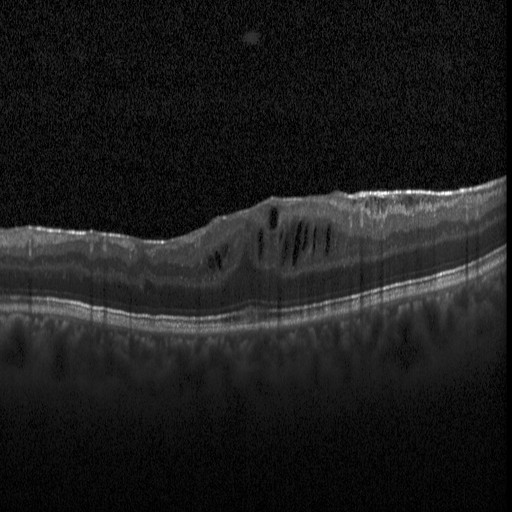
Diagnosis: diabetic macular edema (DME).